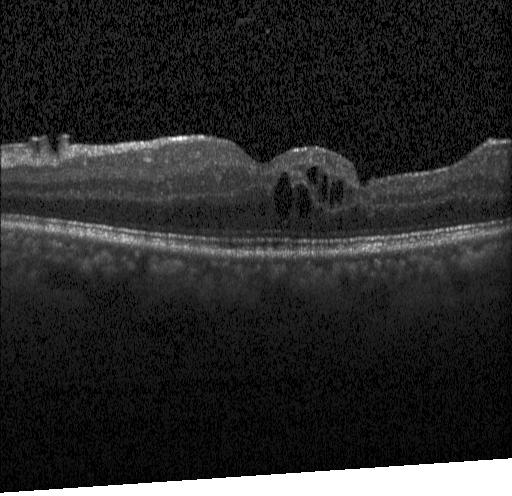

Diagnosis: diabetic macular edema (DME).